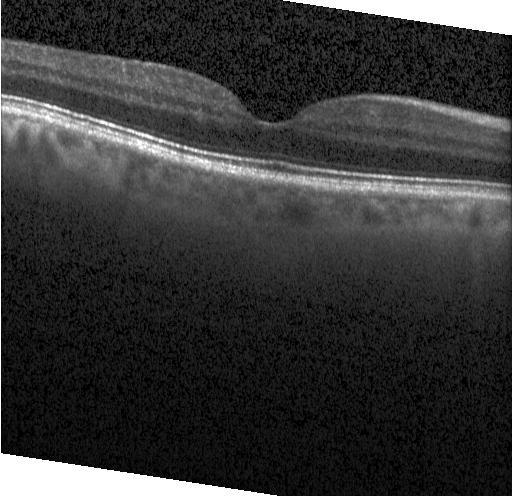 The scan shows no CNV, DME, or drusen.